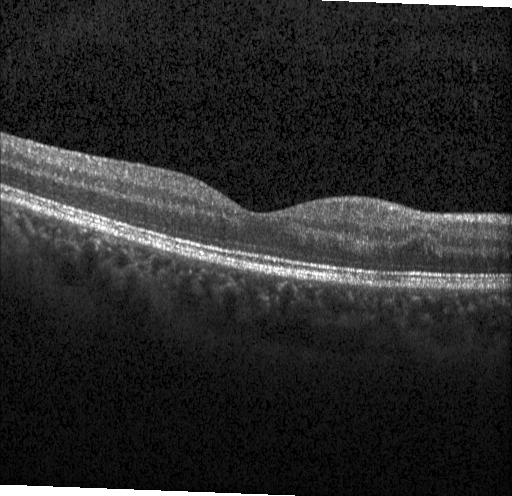

Dx: neither CNV, DME, nor drusen.